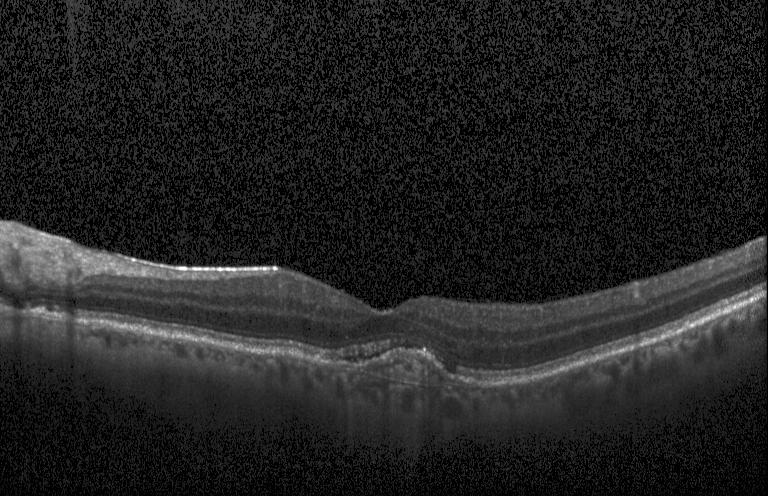
Dx: choroidal neovascularization.